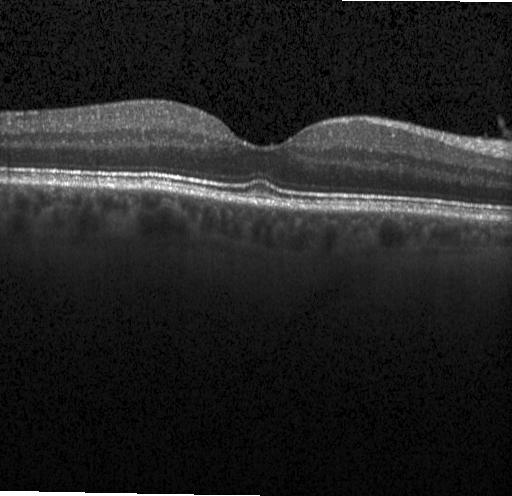

OCT line scan. Diagnosis: neither choroidal neovascularization, diabetic macular edema, nor drusen.